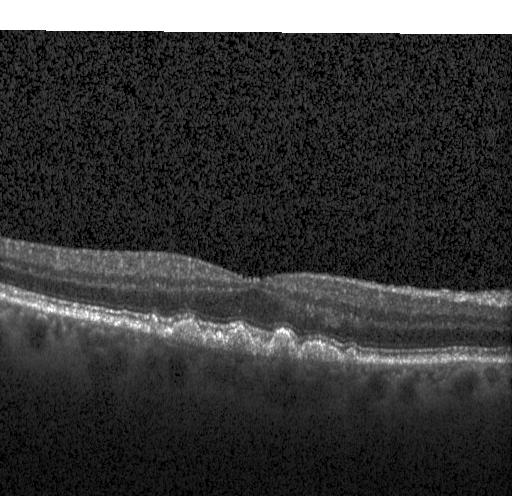

Dx: multiple drusen.